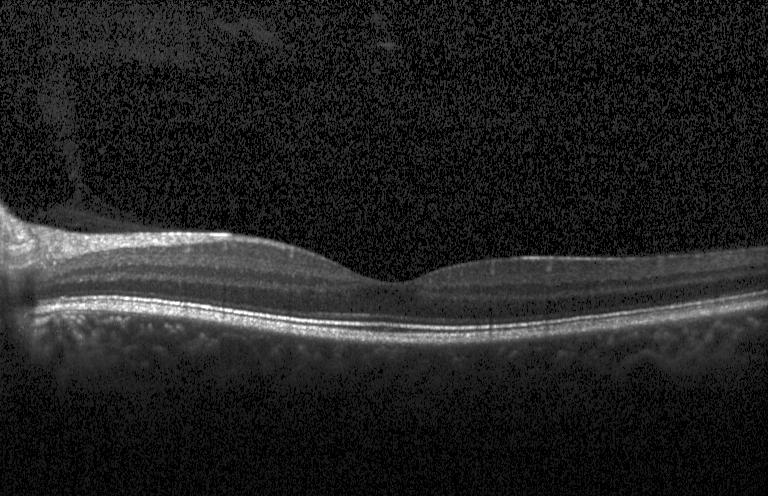 Impression: no evidence of CNV, DME, or drusen.